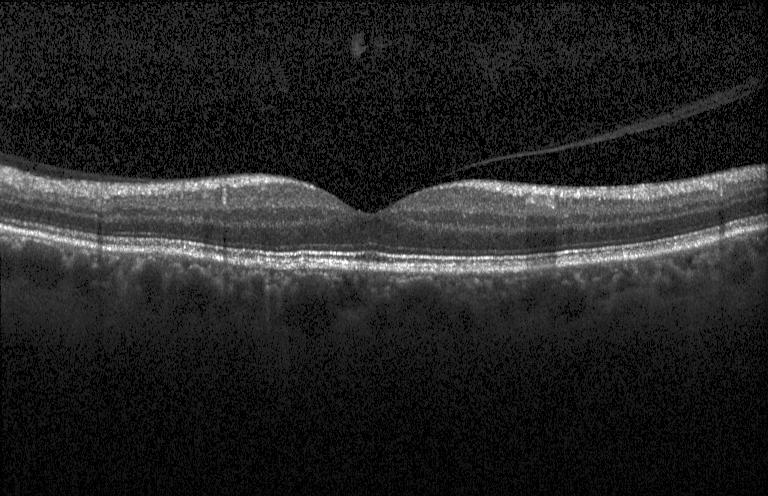 Dx: no CNV, DME, or drusen.